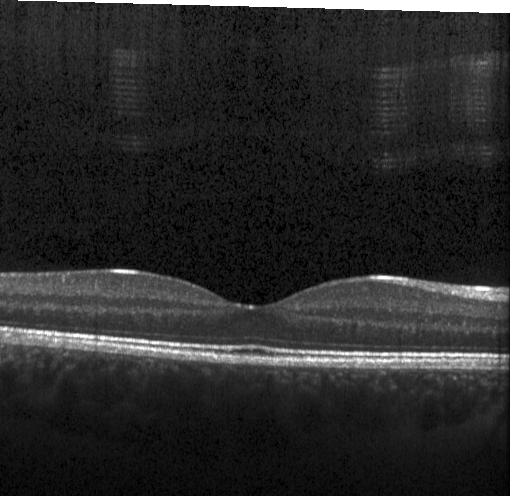

Retinal OCT B-scan
Impression: no choroidal neovascularization, no diabetic macular edema, and no drusen.